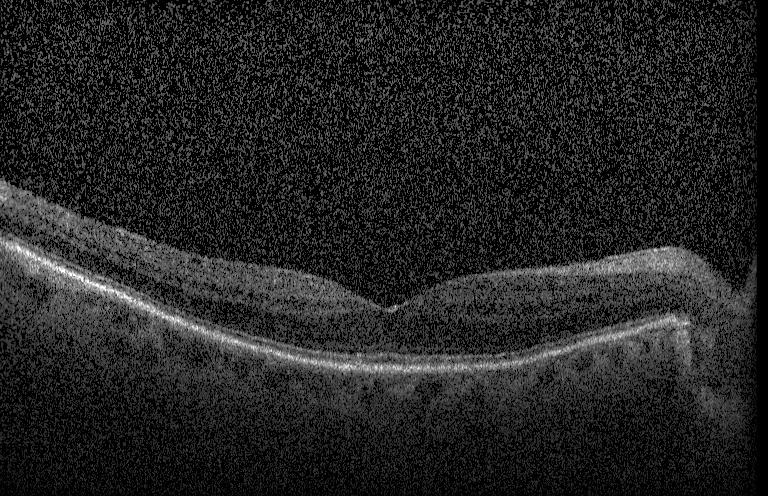
Diagnosis: no CNV, no DME, and no drusen.